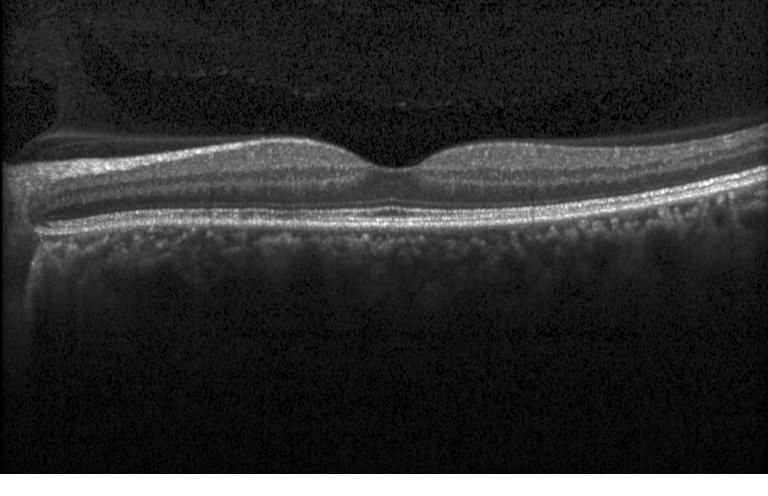 Retinal OCT cross-section.
The scan shows no evidence of choroidal neovascularization, diabetic macular edema, or drusen.